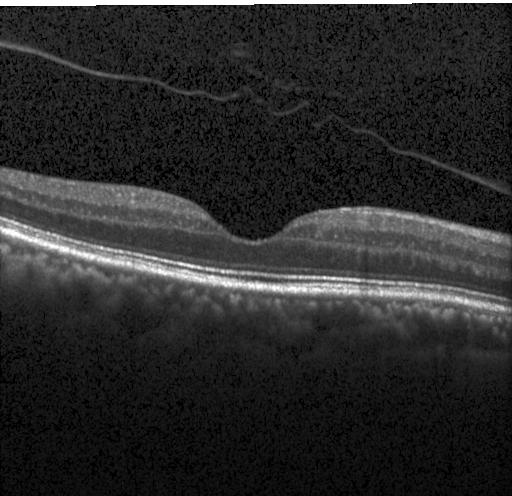
Retinal OCT B-scan; Heidelberg Spectralis OCT system.
Impression: no CNV, DME, or drusen.